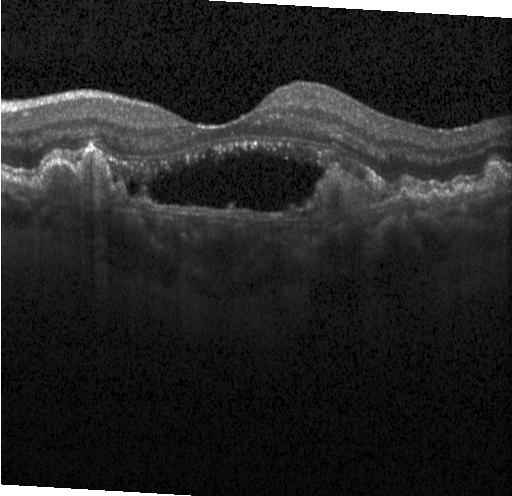

Dx: a choroidal neovascular membrane.